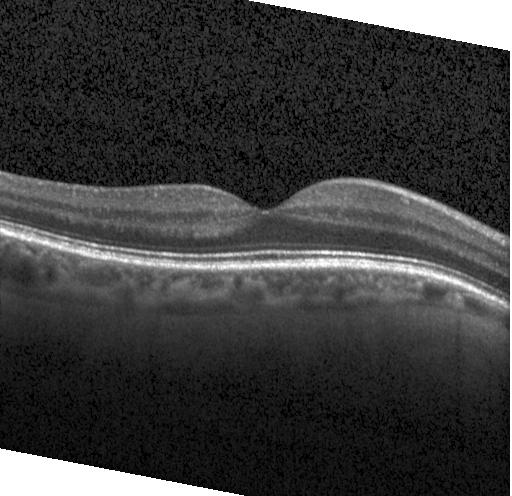

Optical coherence tomography B-scan. Finding: no CNV, no DME, and no drusen.